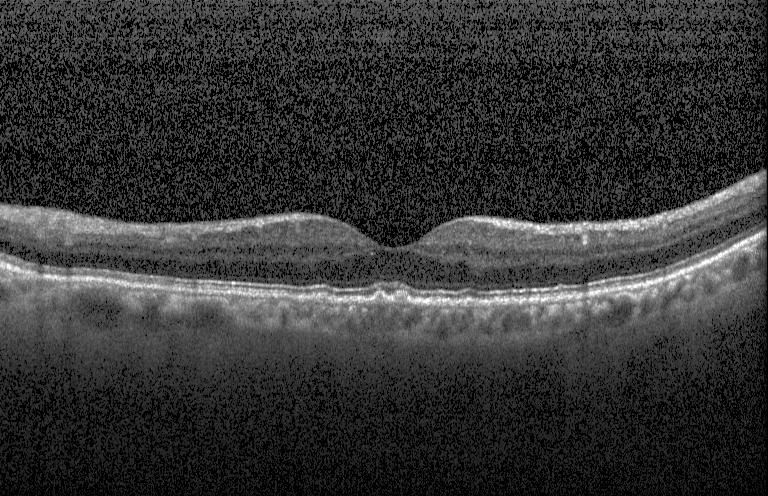
Acquired on a Heidelberg Spectralis. Optical coherence tomography B-scan. Spectral-domain OCT. Horizontal scan through the fovea.
Multiple drusen.